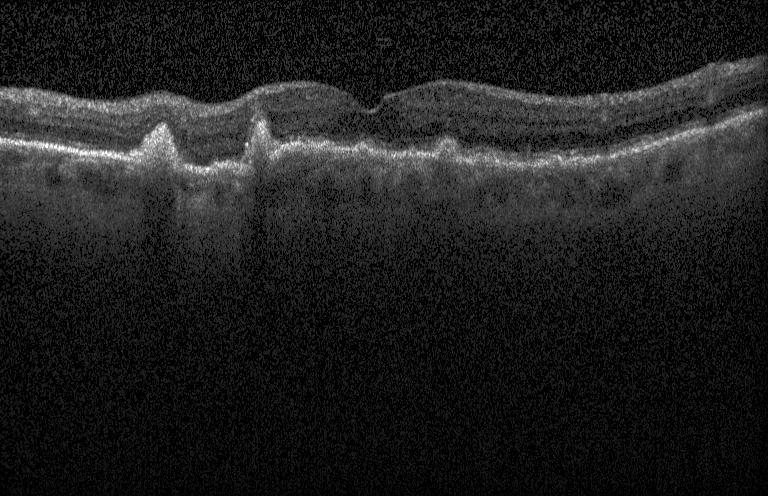
Heidelberg Spectralis. OCT B-scan. Finding: choroidal neovascularization (CNV).